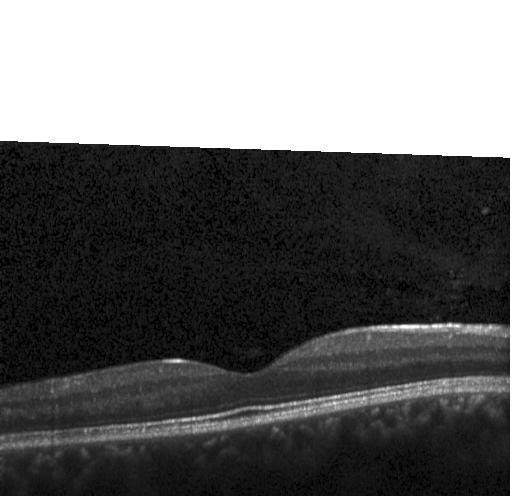 Heidelberg Spectralis OCT system; centered on the fovea; retinal OCT cross-section
Finding: no evidence of choroidal neovascularization, diabetic macular edema, or drusen.